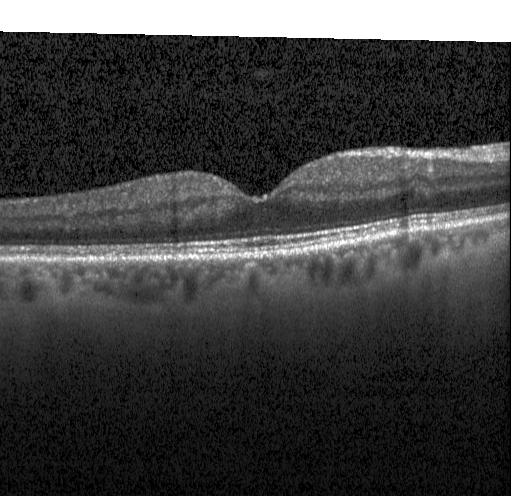 Acquired on a Heidelberg Spectralis · spectral-domain optical coherence tomography · optical coherence tomography scan. OCT finding: no evidence of choroidal neovascularization, diabetic macular edema, or drusen.